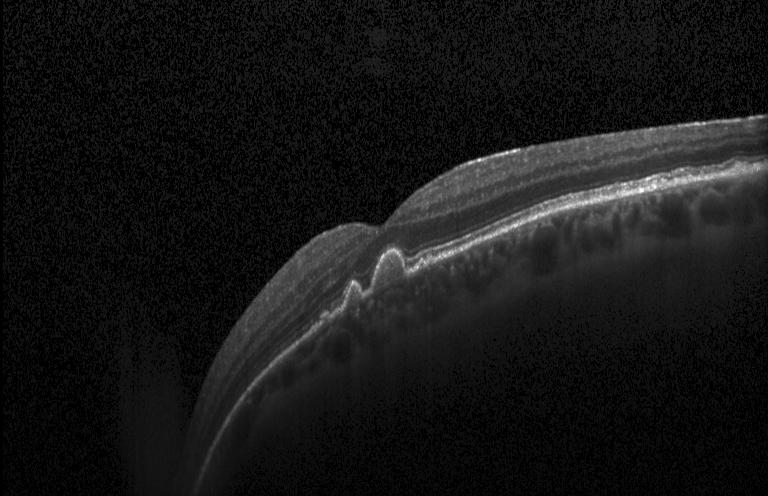
OCT B-scan. Assessment: multiple drusen.